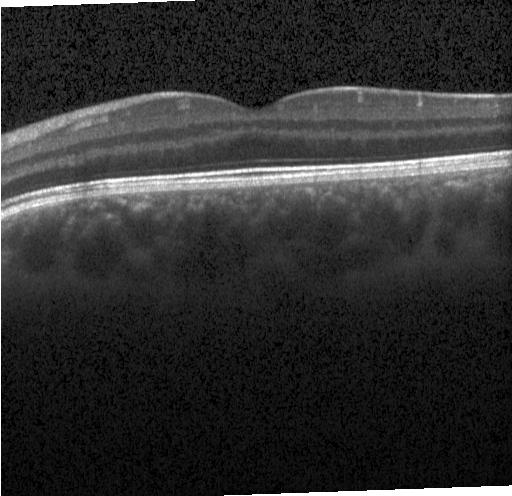
Horizontal scan through the fovea, optical coherence tomography scan
The scan shows neither CNV, DME, nor drusen.